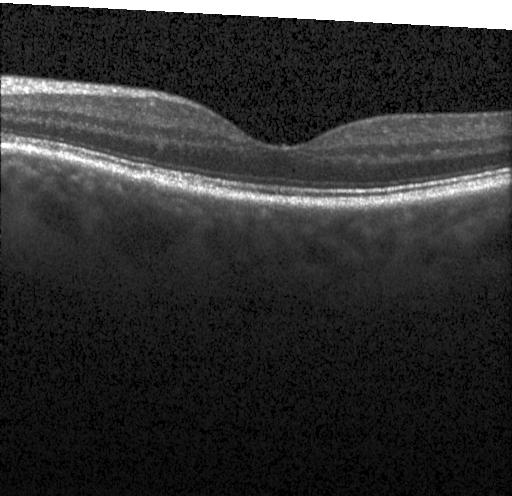 Retinal OCT B-scan. Macular scan. Instrument: Heidelberg Spectralis. Spectral-domain optical coherence tomography — Finding: no choroidal neovascularization, diabetic macular edema, or drusen.